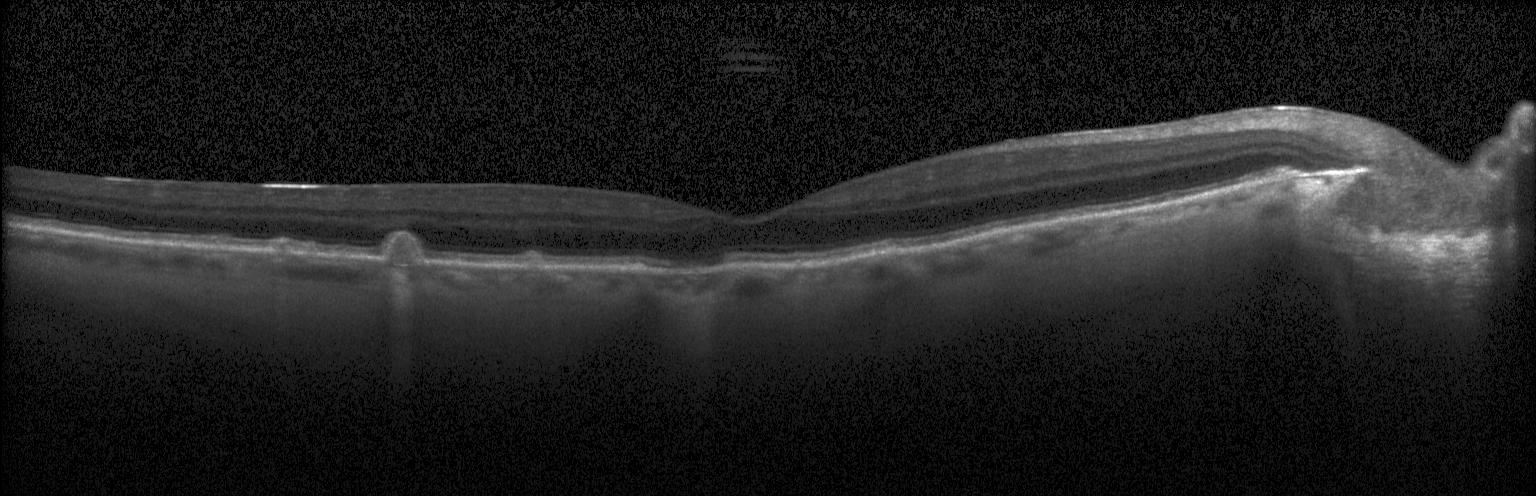

OCT scan showing sub-RPE drusenoid deposits.